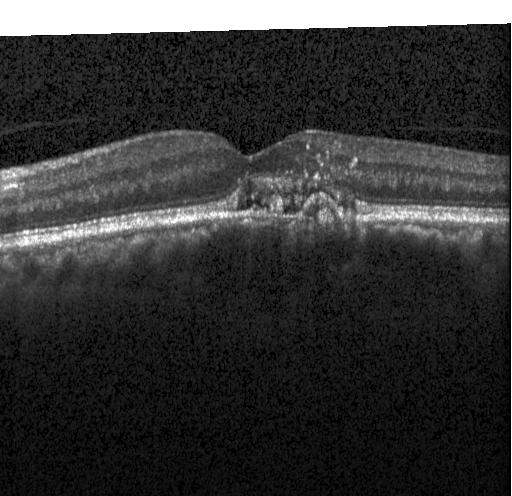 OCT finding: choroidal neovascularization.